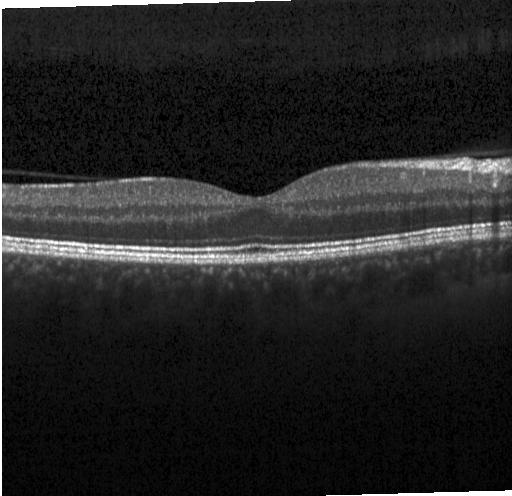
Retinal OCT cross-section; Heidelberg Spectralis; fovea-centered; SD-OCT. Assessment: neither CNV, DME, nor drusen.